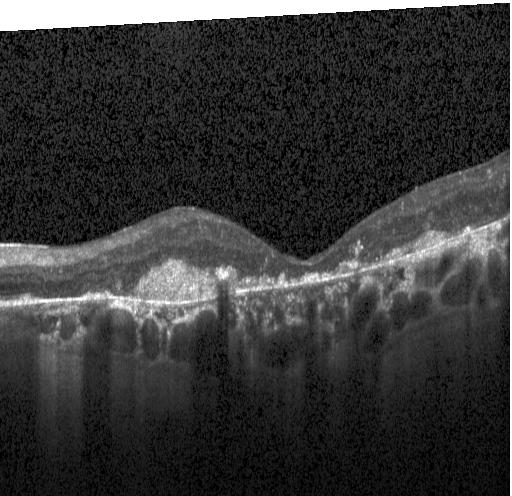

The scan shows a choroidal neovascular membrane.